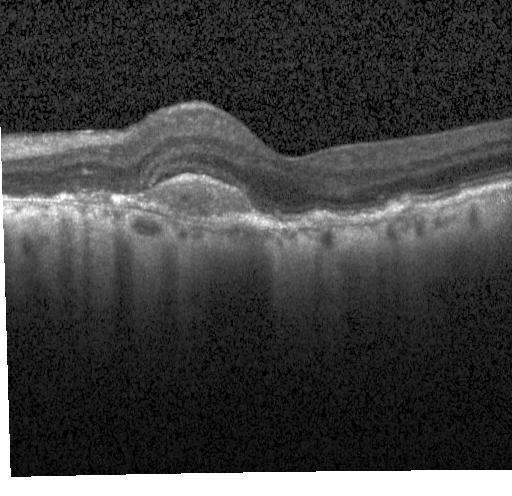

OCT line scan · SD-OCT · acquired on a Heidelberg Spectralis · macular scan.
Impression: choroidal neovascularization.